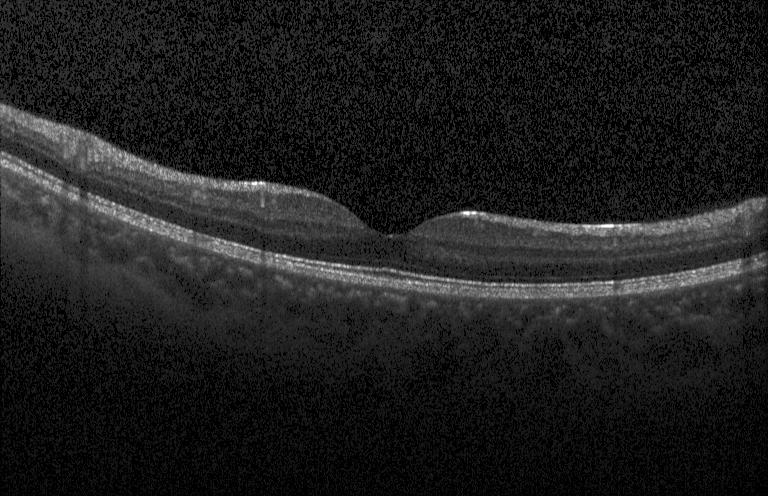
Impression: no choroidal neovascularization, diabetic macular edema, or drusen.